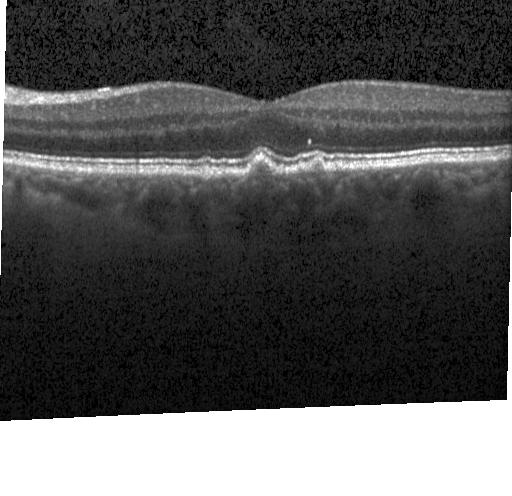
OCT B-scan showing drusen.